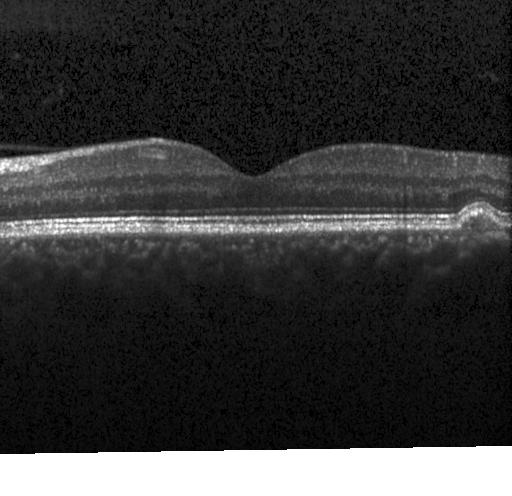
Impression: sub-RPE drusenoid deposits.